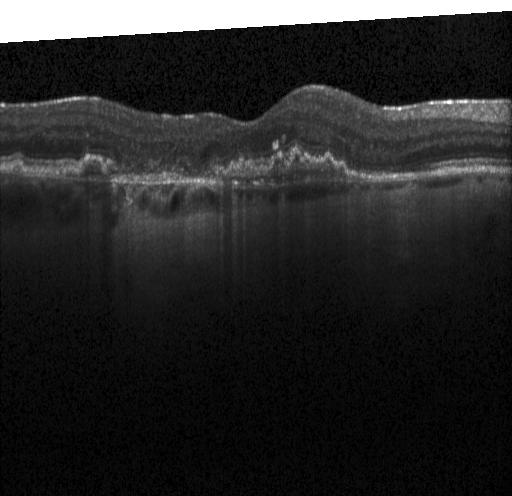 Retinal OCT B-scan
Impression: a choroidal neovascular membrane.